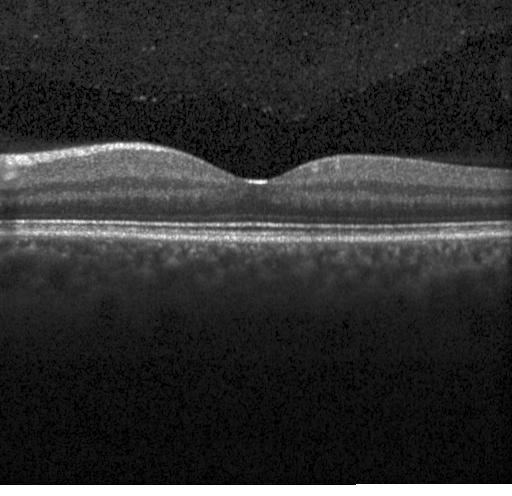

Impression: no choroidal neovascularization, diabetic macular edema, or drusen.